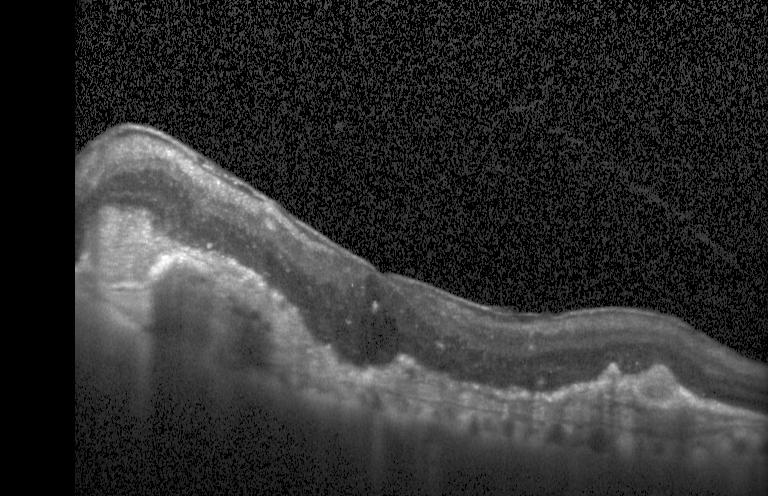

Centered on the fovea. Acquired on a Heidelberg Spectralis. Retinal OCT B-scan. SD-OCT
OCT finding: choroidal neovascularization (CNV).